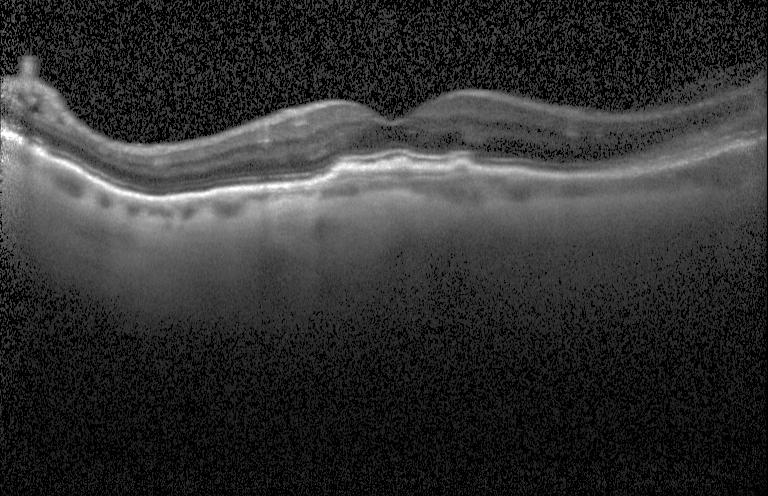

Acquired on a Heidelberg Spectralis. Through the macula. Spectral-domain optical coherence tomography. Optical coherence tomography B-scan
Diagnosis: a choroidal neovascular membrane.